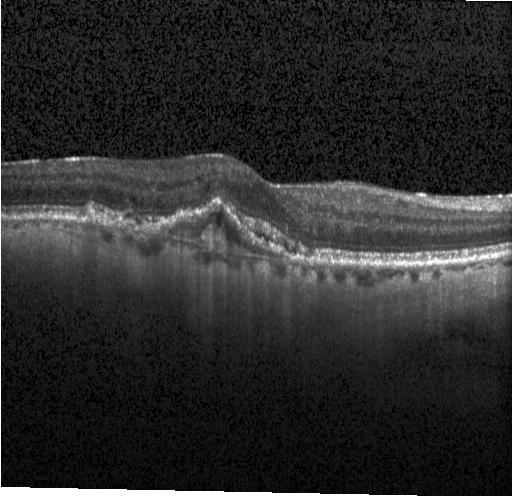 Retinal OCT cross-section, macular scan — Impression: a choroidal neovascular membrane.